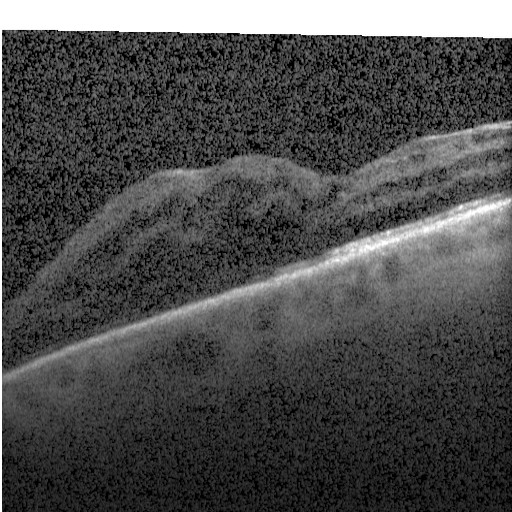
Retinal OCT cross-section
Impression: diabetic macular edema (DME).